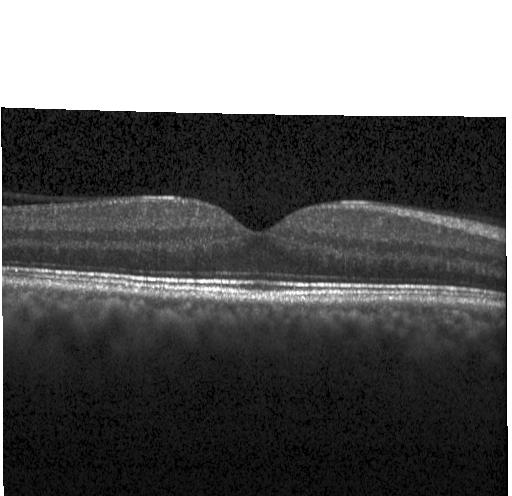 OCT B-scan — Finding: no evidence of CNV, DME, or drusen.